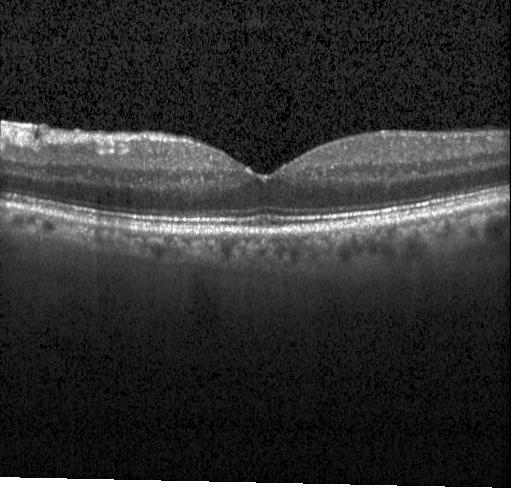

OCT finding: no evidence of CNV, DME, or drusen.